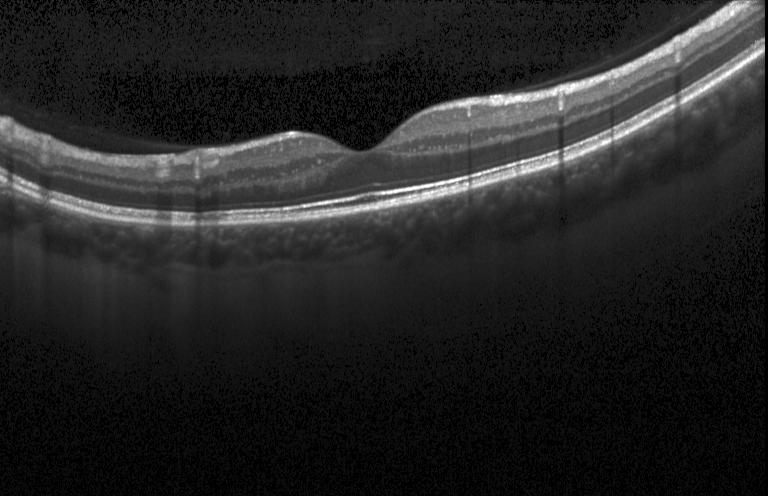

Optical coherence tomography scan. Diagnosis: neither choroidal neovascularization, diabetic macular edema, nor drusen.